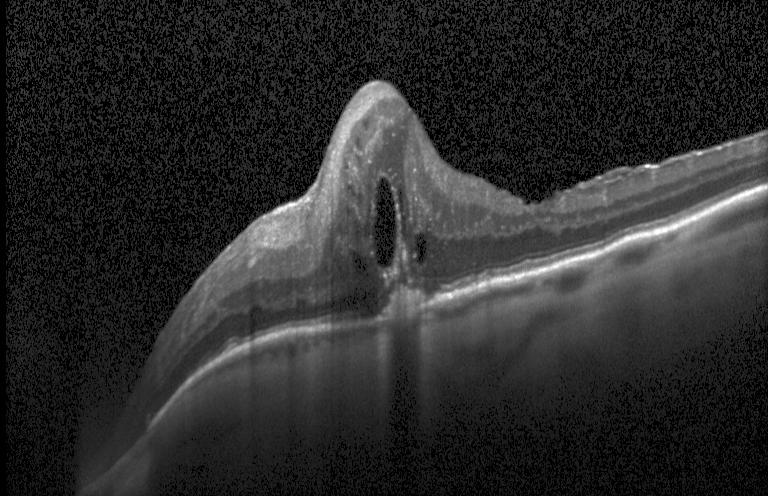

Fovea-centered, acquired on a Heidelberg Spectralis, OCT B-scan — A choroidal neovascular membrane.